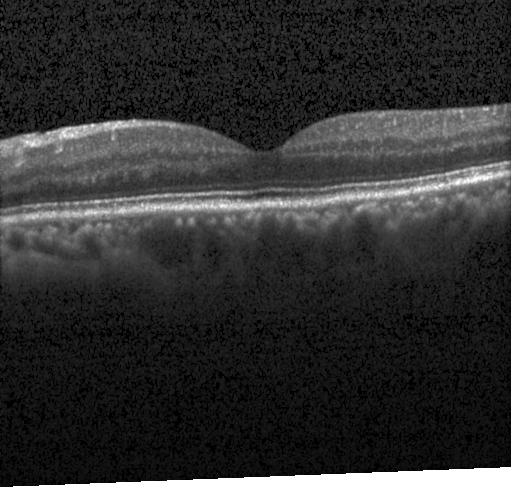

Optical coherence tomography B-scan. Through the macula. Heidelberg Spectralis — No choroidal neovascularization, no diabetic macular edema, and no drusen.